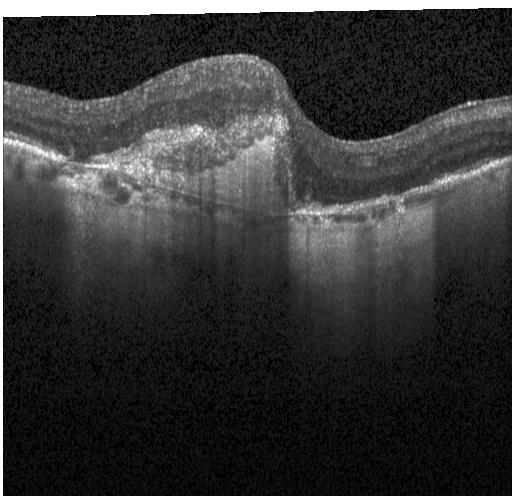 Impression: CNV.